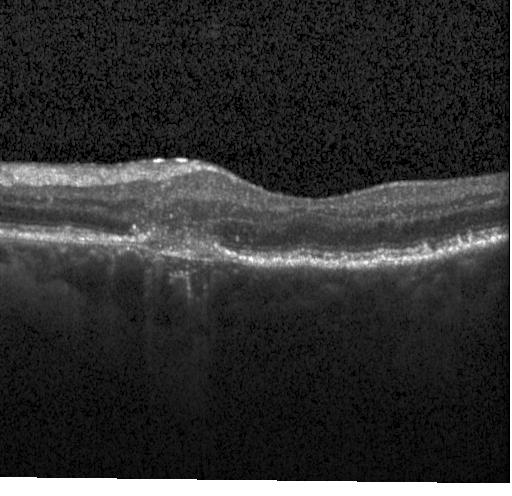 Macular scan · instrument: Heidelberg Spectralis · retinal OCT cross-section — Finding: CNV.